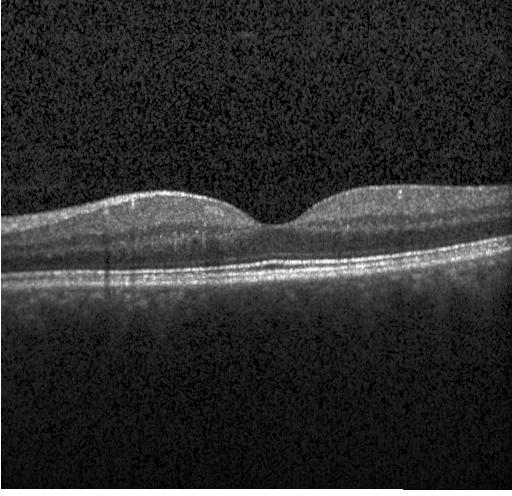
Impression: no choroidal neovascularization, diabetic macular edema, or drusen.